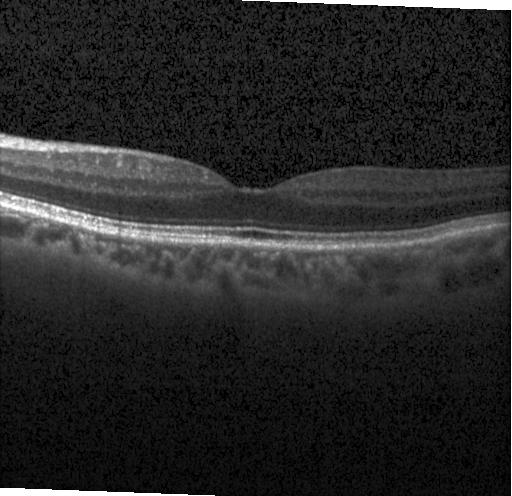
Optical coherence tomography B-scan, horizontal scan through the fovea, spectral-domain optical coherence tomography, Heidelberg Spectralis — No CNV, no DME, and no drusen.